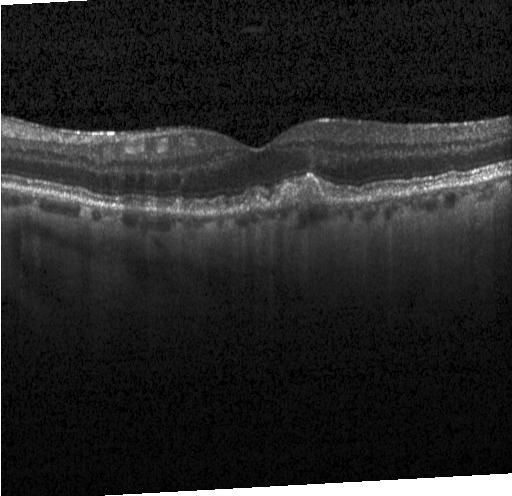

Finding: sub-RPE drusenoid deposits.